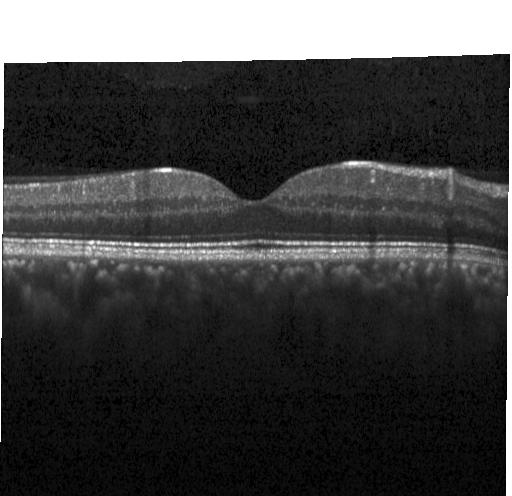

Macular OCT: no evidence of choroidal neovascularization, diabetic macular edema, or drusen.